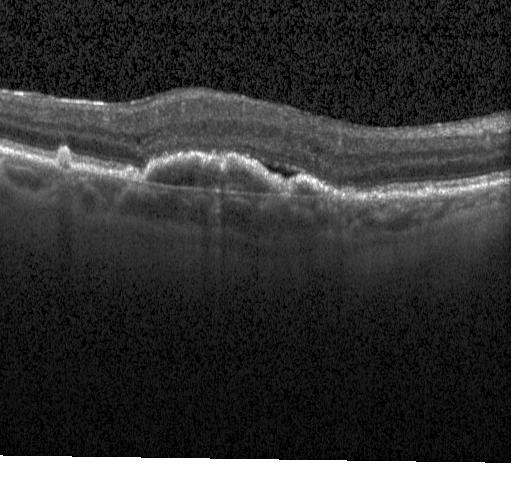

OCT scan showing a choroidal neovascular membrane.